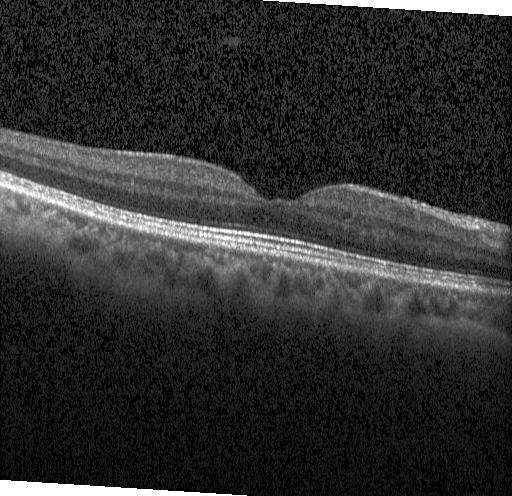 Spectral-domain OCT, retinal OCT cross-section — Finding: no CNV, no DME, and no drusen.